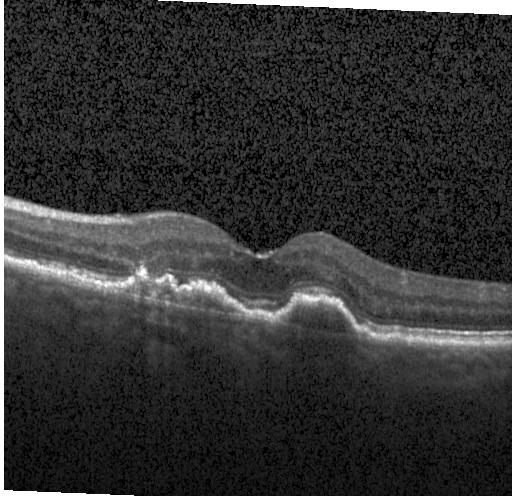 Impression: choroidal neovascularization (CNV).